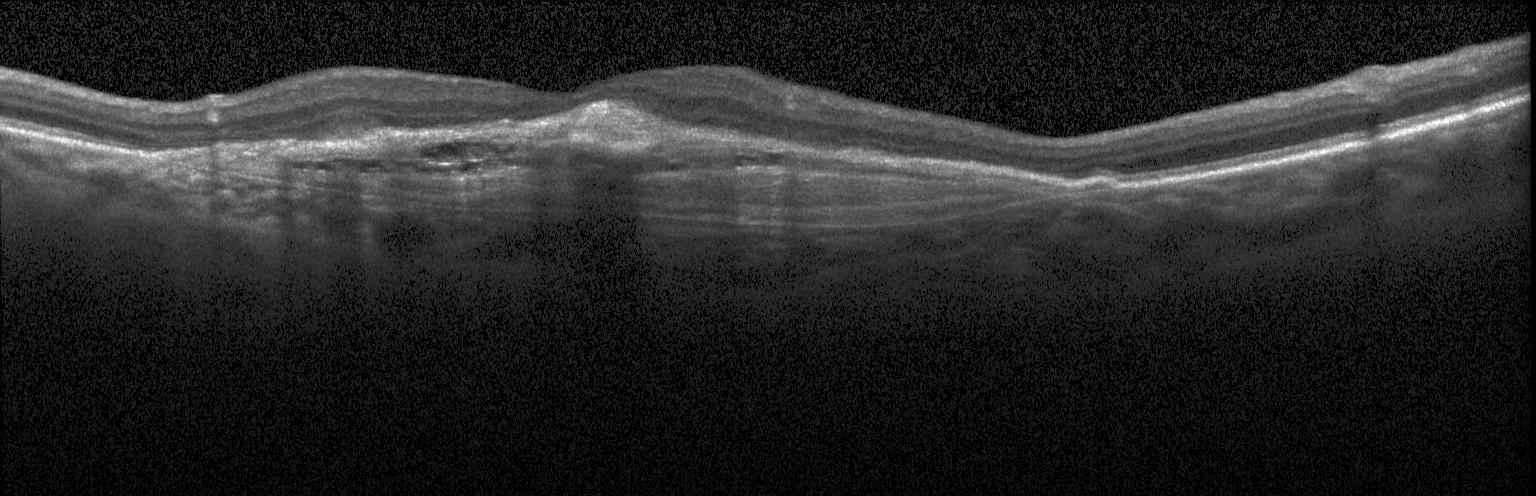 Retinal OCT B-scan, spectral-domain OCT, Heidelberg Spectralis OCT system, centered on the fovea. Impression: choroidal neovascularization.